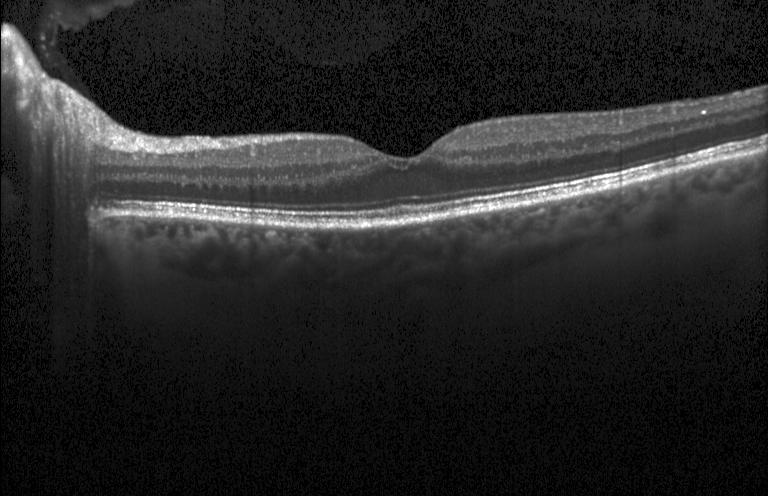 Dx: no CNV, DME, or drusen.